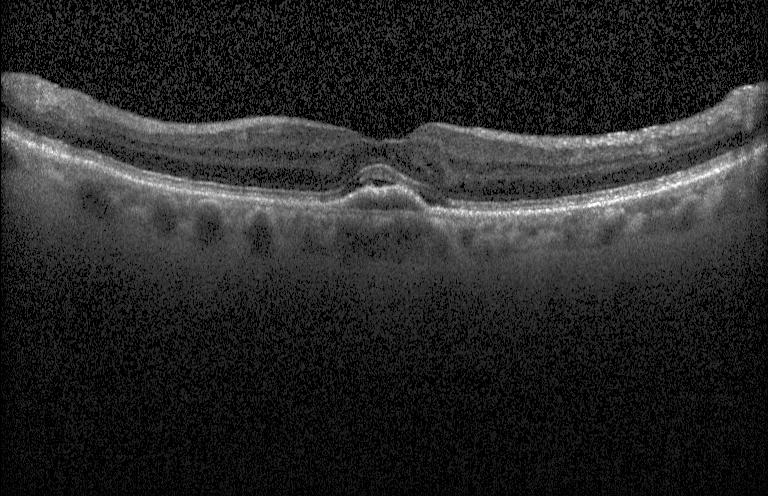 Retinal OCT B-scan. Heidelberg Spectralis.
Finding: a choroidal neovascular membrane.